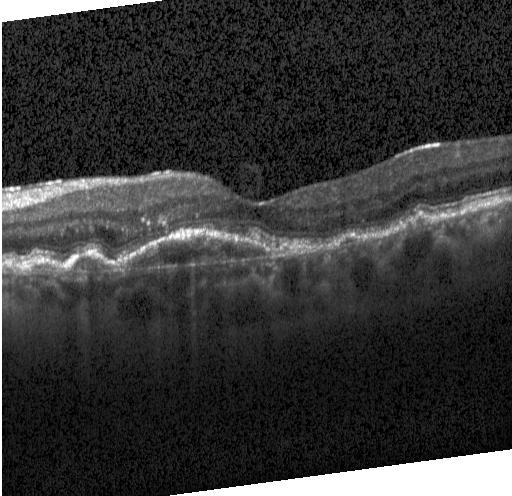 Retinal OCT cross-section. SD-OCT. Heidelberg Spectralis
Finding: choroidal neovascularization (CNV).